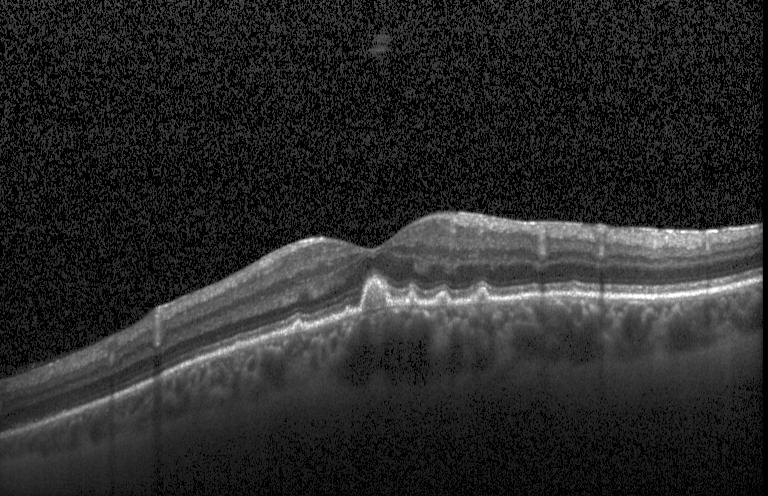

Optical coherence tomography scan — Dx: sub-RPE drusenoid deposits.